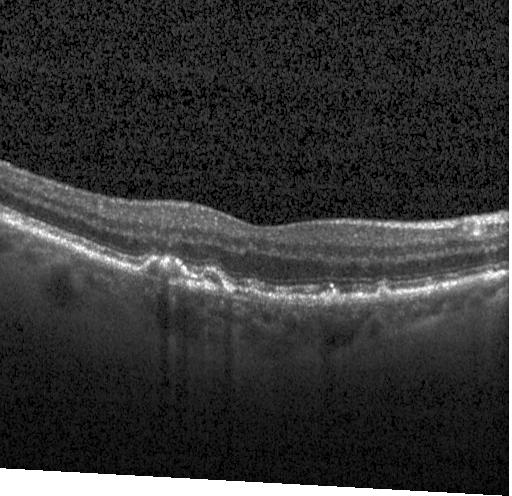
SD-OCT. Heidelberg Spectralis OCT system. OCT B-scan. Fovea-centered — Diagnosis: multiple drusen.